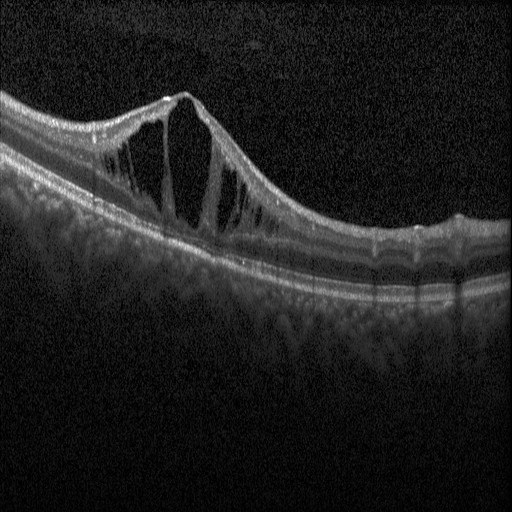
The scan shows diabetic macular edema.